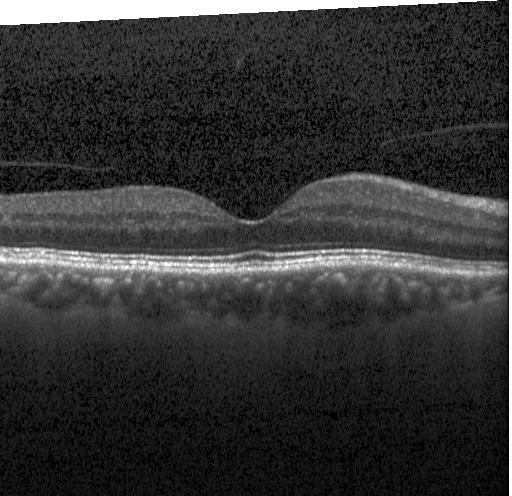
Diagnosis: neither CNV, DME, nor drusen.